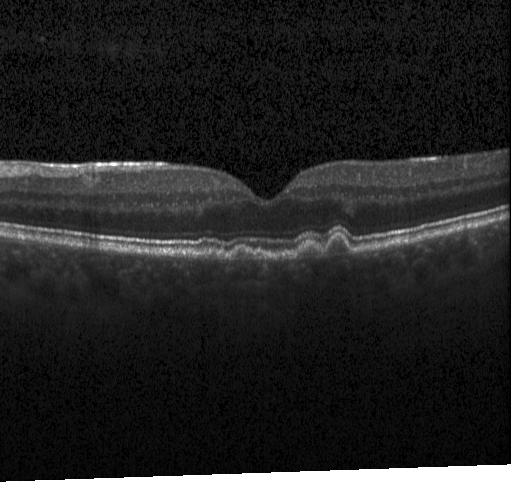 Retinal OCT cross-section, Heidelberg Spectralis, centered on the fovea, spectral-domain OCT.
Dx: multiple drusen.